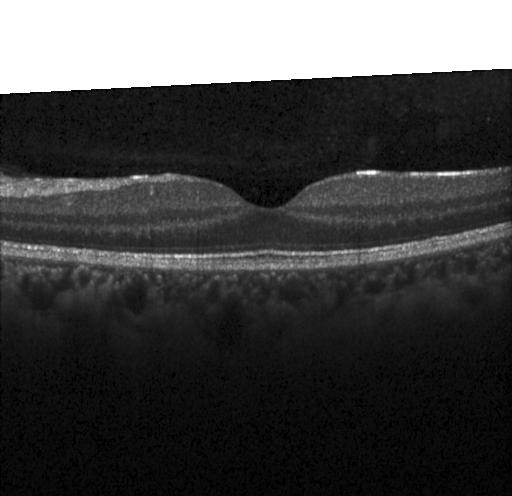

Optical coherence tomography B-scan, Heidelberg Spectralis, spectral-domain optical coherence tomography.
This B-scan demonstrates no CNV, no DME, and no drusen.